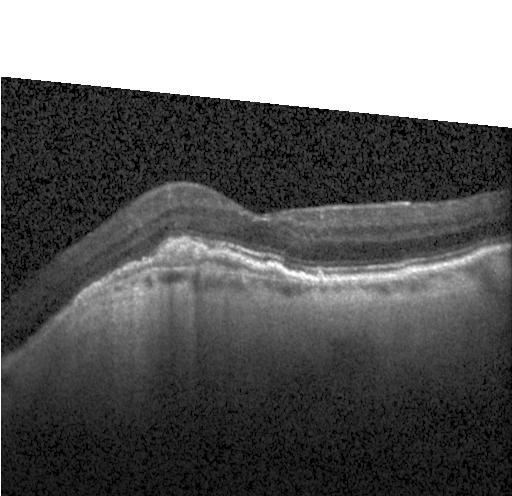 Diagnosis: choroidal neovascularization.